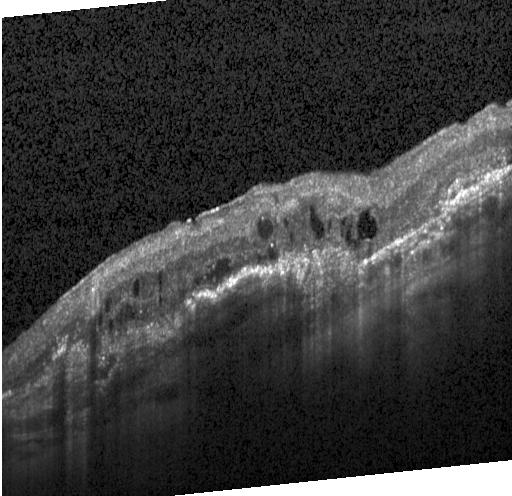
Instrument: Heidelberg Spectralis · OCT B-scan · SD-OCT. Impression: a choroidal neovascular membrane.